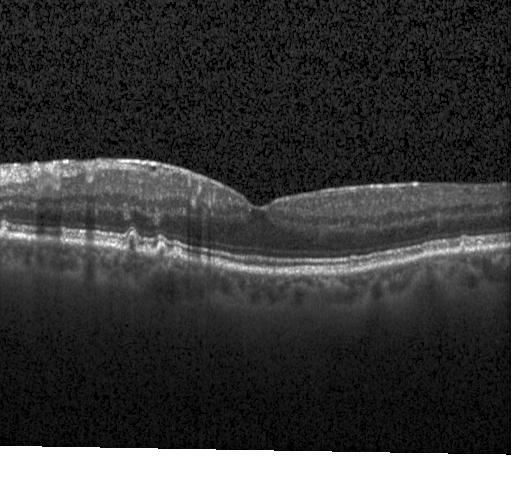
Finding: sub-RPE drusenoid deposits.